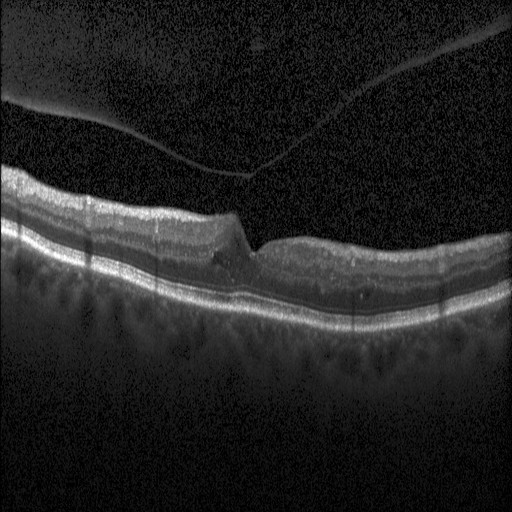
Retinal OCT cross-section · acquired on a Heidelberg Spectralis · spectral-domain OCT · macular scan.
Dx: diabetic macular edema.